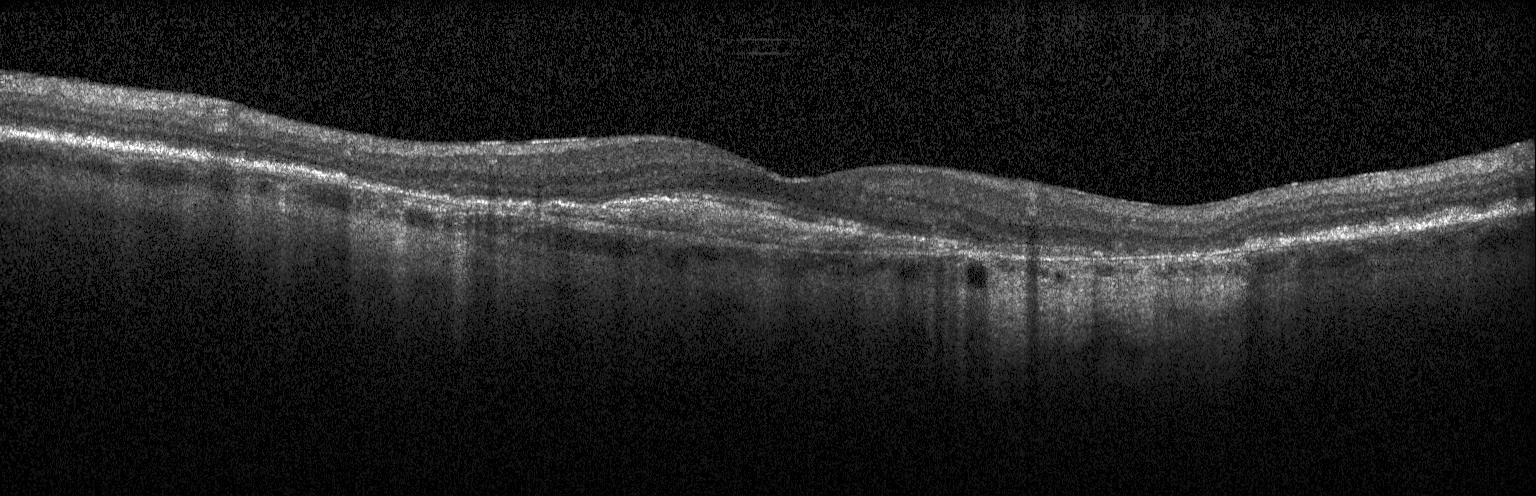

Optical coherence tomography scan, spectral-domain OCT. Diagnosis: CNV.